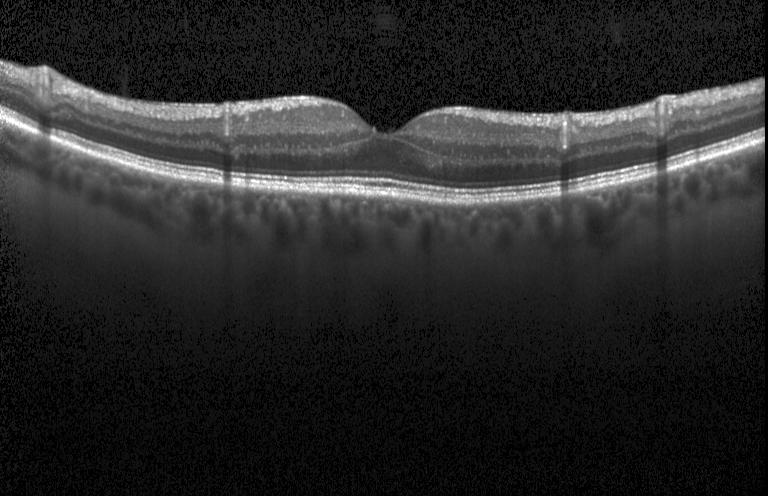

Finding: no CNV, no DME, and no drusen.